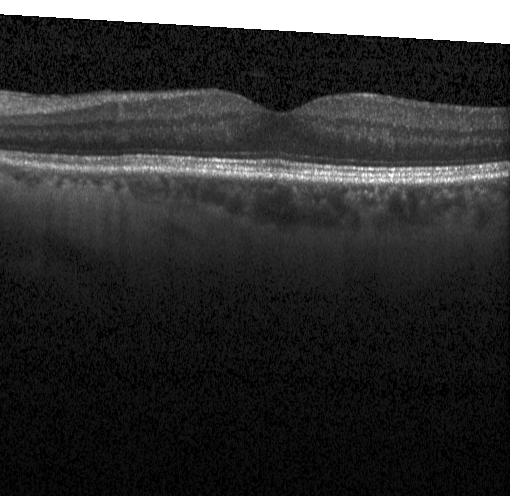

OCT finding: neither choroidal neovascularization, diabetic macular edema, nor drusen.